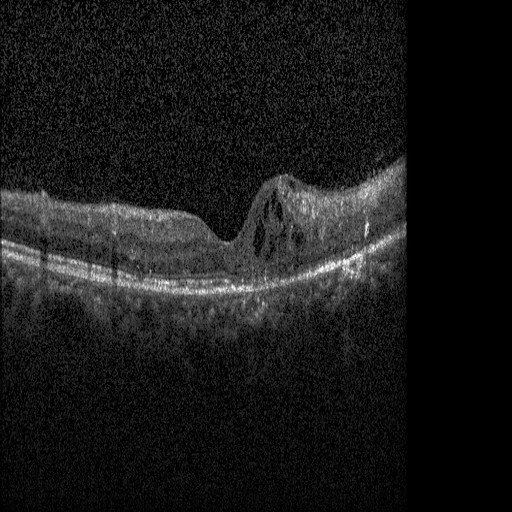
Diagnosis: diabetic macular edema.